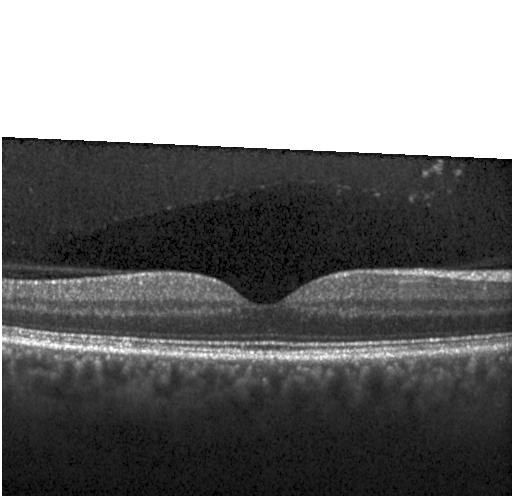 Fovea-centered, instrument: Heidelberg Spectralis, retinal OCT cross-section
Diagnosis: neither choroidal neovascularization, diabetic macular edema, nor drusen.